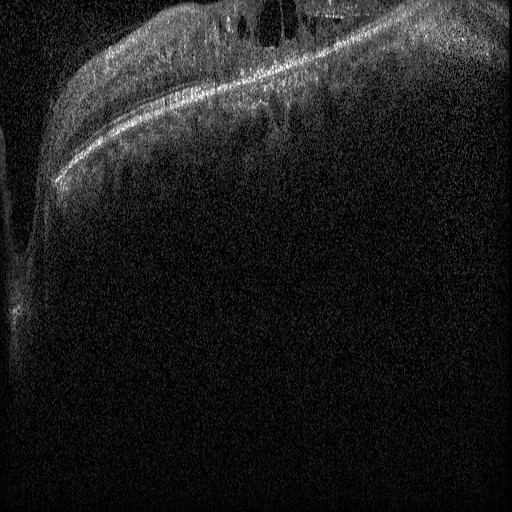
Retinal OCT cross-section
OCT finding: diabetic macular edema.